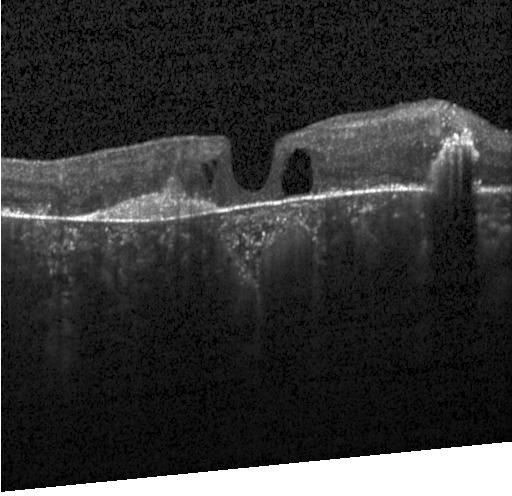

Diagnosis: choroidal neovascularization (CNV).